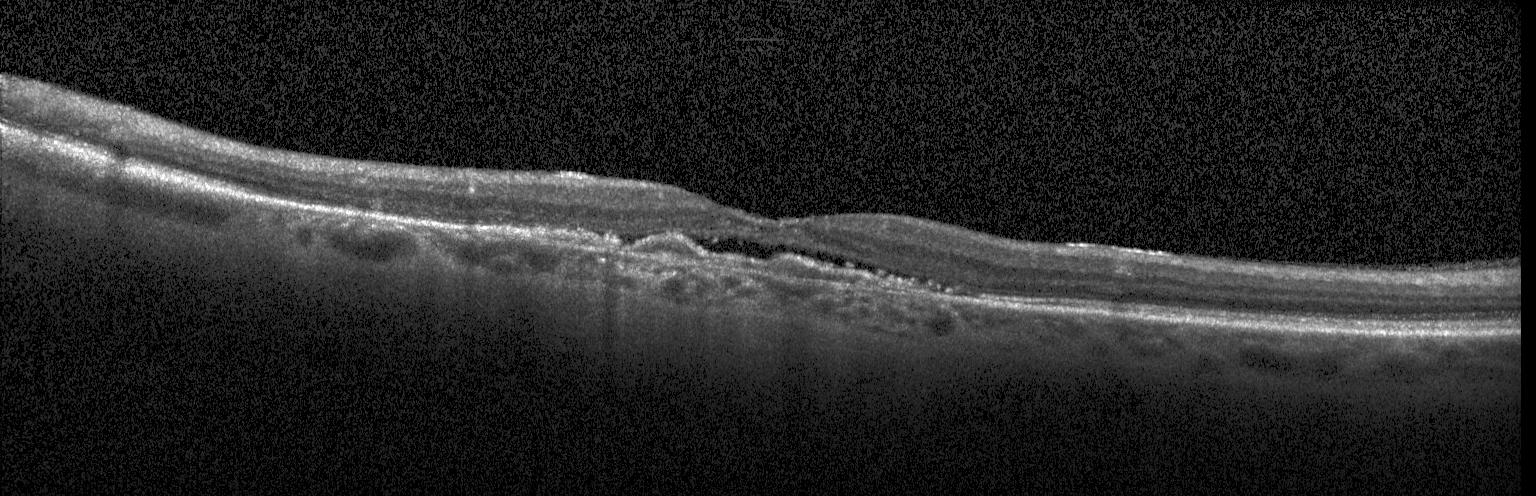 Through the macula, OCT B-scan.
Dx: a choroidal neovascular membrane.